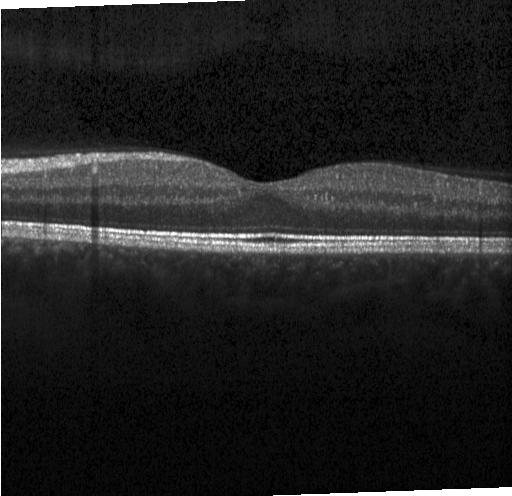

Spectral-domain optical coherence tomography; OCT line scan; instrument: Heidelberg Spectralis; macular scan — Finding: no choroidal neovascularization, no diabetic macular edema, and no drusen.